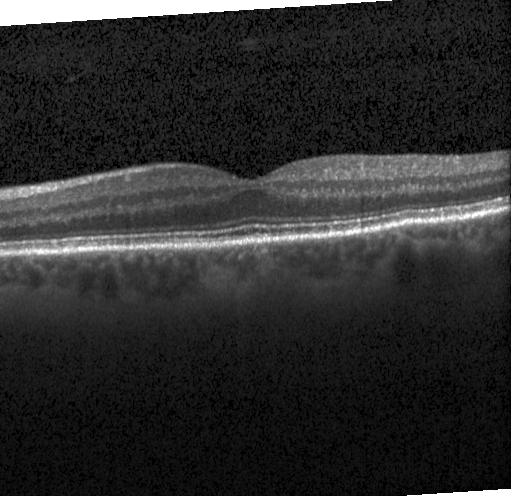 Instrument: Heidelberg Spectralis. Retinal OCT B-scan. Horizontal scan through the fovea. SD-OCT. Diagnosis: no evidence of CNV, DME, or drusen.